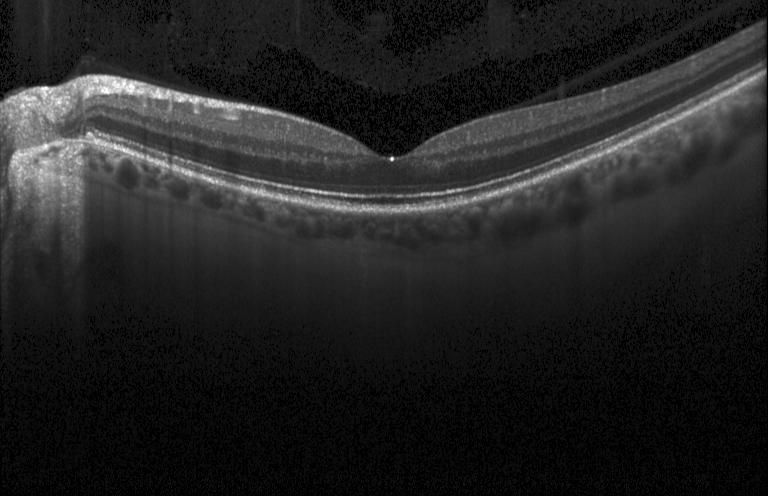 Spectral-domain OCT. Instrument: Heidelberg Spectralis. Optical coherence tomography scan.
No CNV, DME, or drusen.